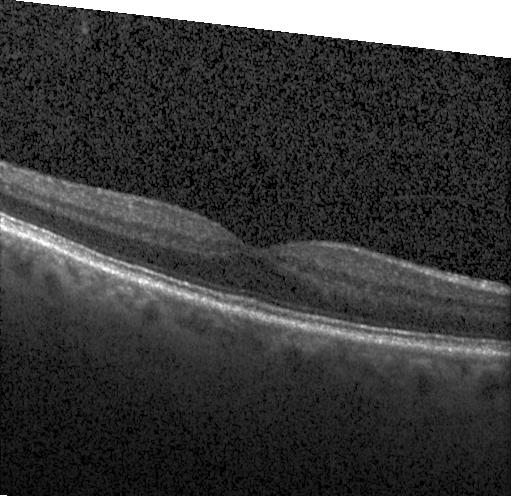 Optical coherence tomography scan, acquired on a Heidelberg Spectralis, SD-OCT.
Neither choroidal neovascularization, diabetic macular edema, nor drusen.